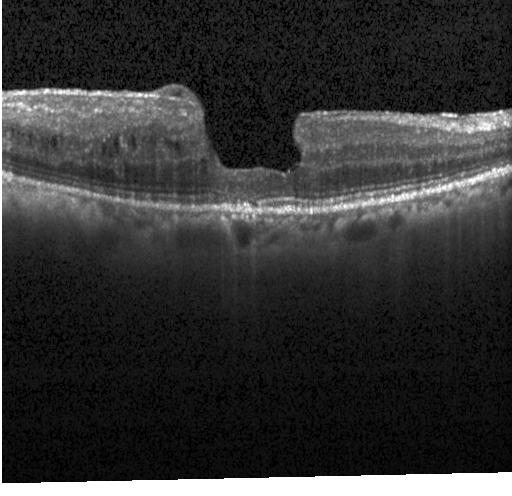
Retinal OCT cross-section. Horizontal scan through the fovea. Acquired on a Heidelberg Spectralis.
Diabetic macular edema.